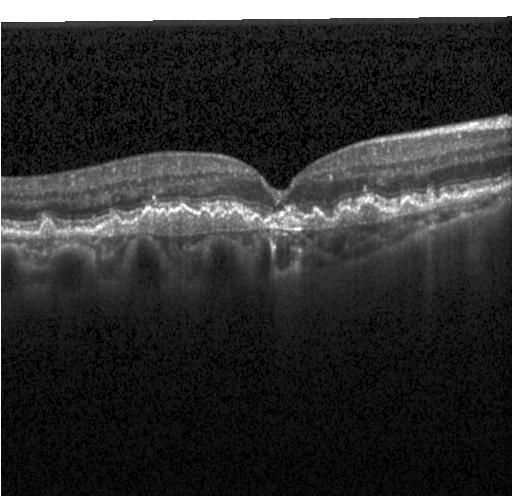 Spectral-domain optical coherence tomography. OCT B-scan. The scan shows a choroidal neovascular membrane.